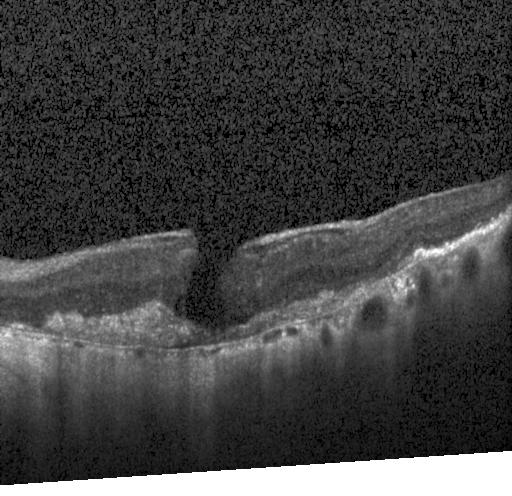
Heidelberg Spectralis OCT system · OCT line scan.
A choroidal neovascular membrane.